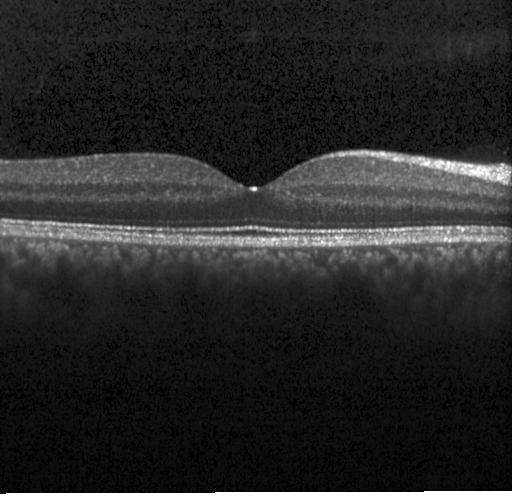 Macular OCT demonstrating no CNV, DME, or drusen.